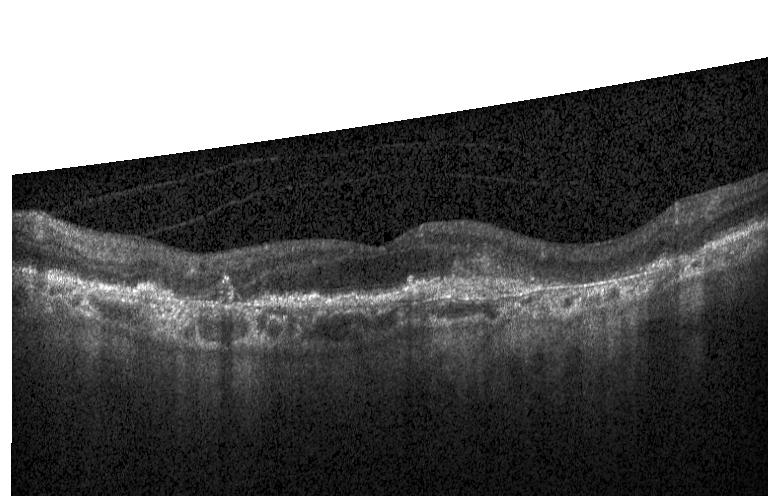 Assessment: choroidal neovascularization.